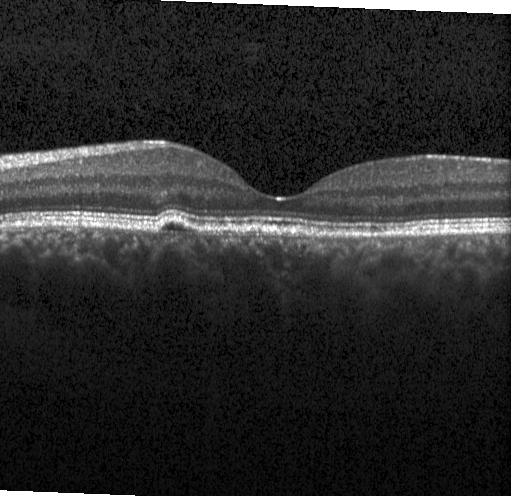 OCT scan showing drusen.